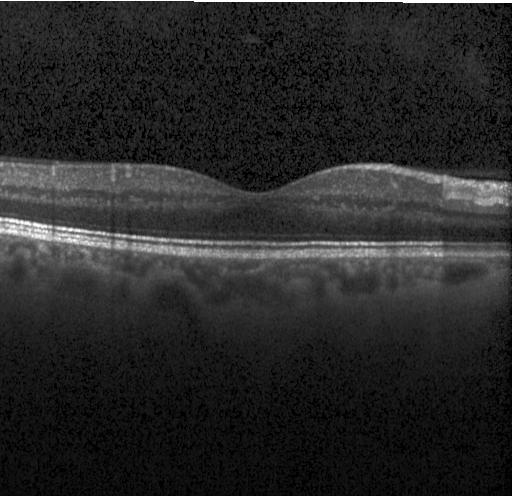
Spectral-domain optical coherence tomography, retinal OCT B-scan.
Impression: no evidence of CNV, DME, or drusen.